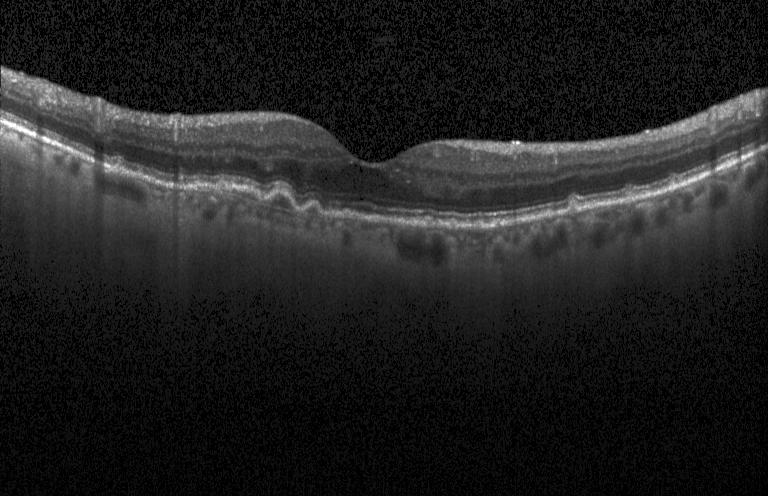
SD-OCT; fovea-centered; retinal OCT B-scan
This B-scan demonstrates multiple drusen.